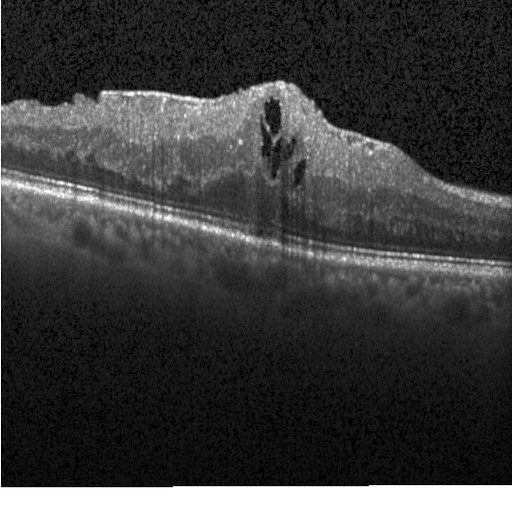 SD-OCT, fovea-centered, instrument: Heidelberg Spectralis, optical coherence tomography B-scan — Impression: diabetic macular edema.